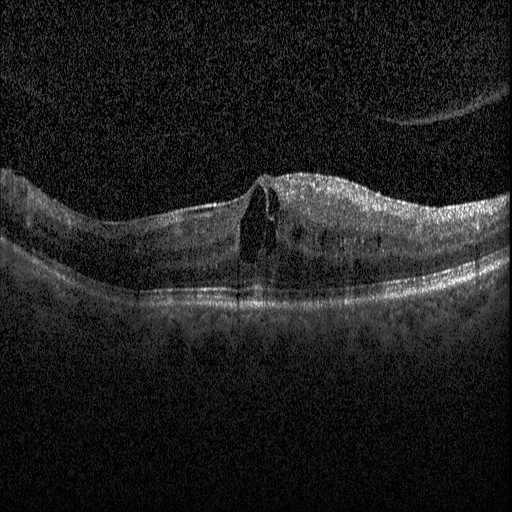

Diabetic macular edema.